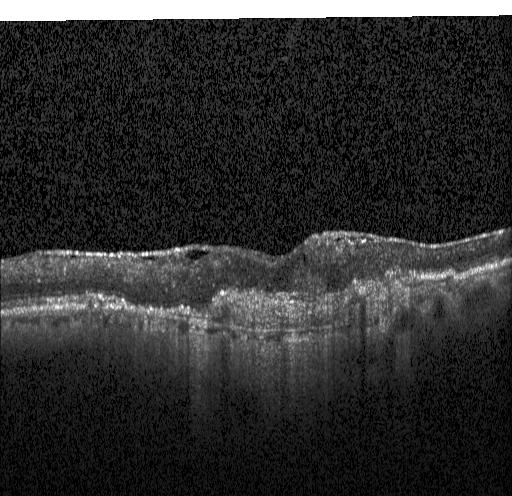 SD-OCT, optical coherence tomography B-scan, Heidelberg Spectralis OCT system, macular scan — Finding: a choroidal neovascular membrane.